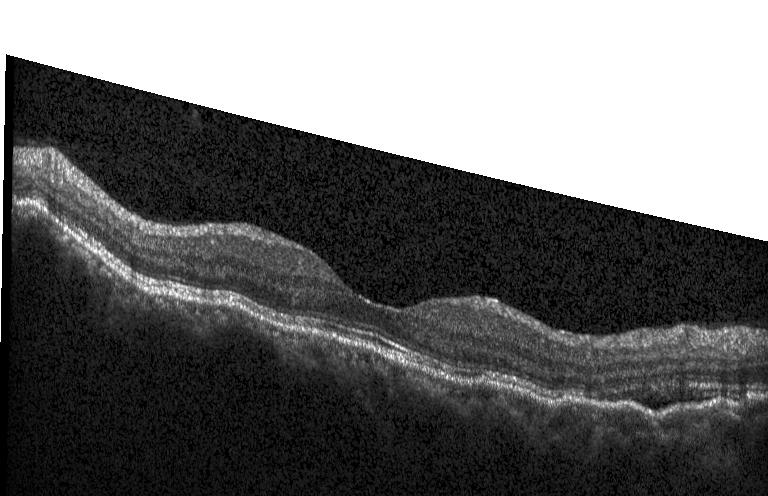 Retinal OCT B-scan · spectral-domain optical coherence tomography.
Assessment: CNV.